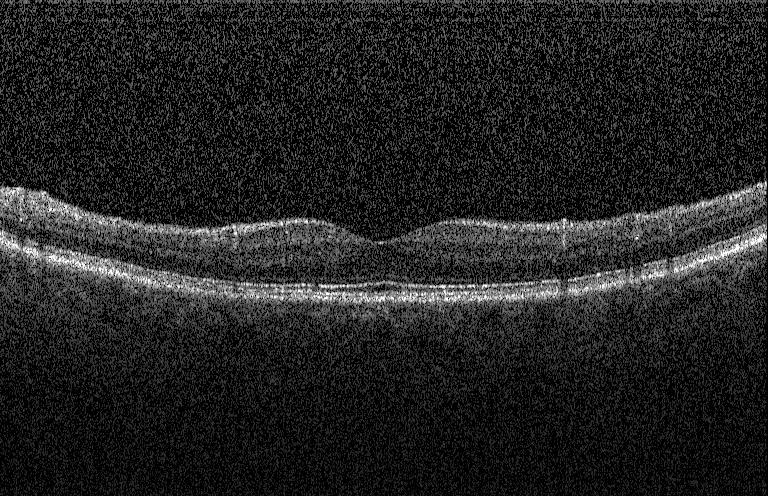 SD-OCT · centered on the fovea · instrument: Heidelberg Spectralis · OCT B-scan.
Macular OCT: no CNV, no DME, and no drusen.